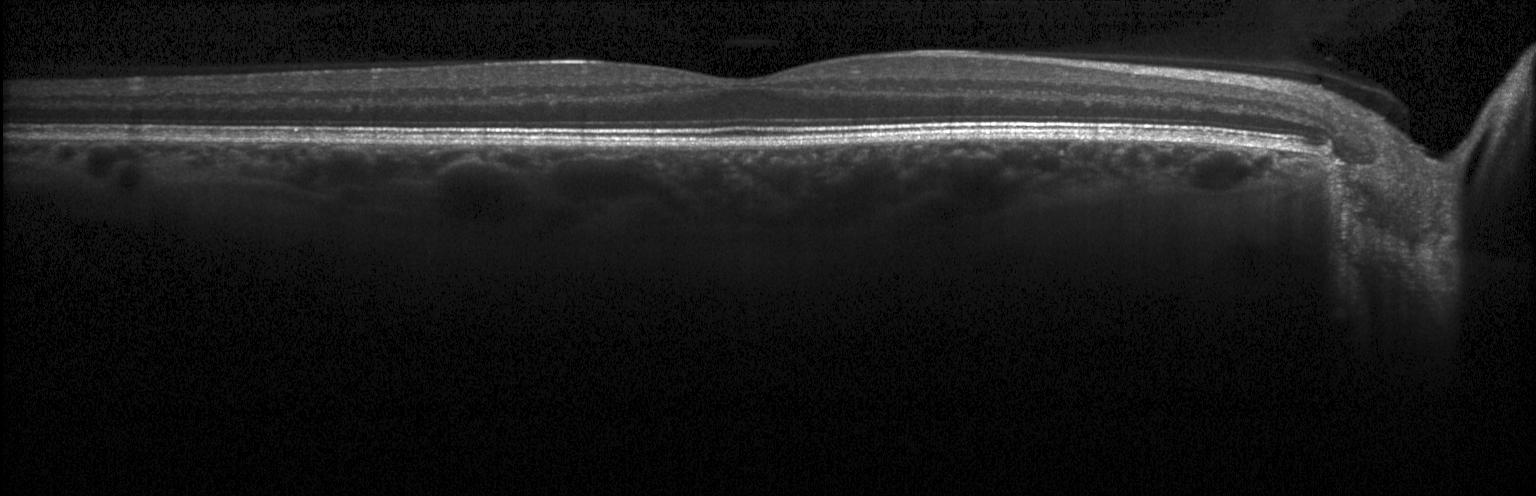

Retinal OCT cross-section. Spectral-domain OCT. Instrument: Heidelberg Spectralis
Diagnosis: no choroidal neovascularization, diabetic macular edema, or drusen.